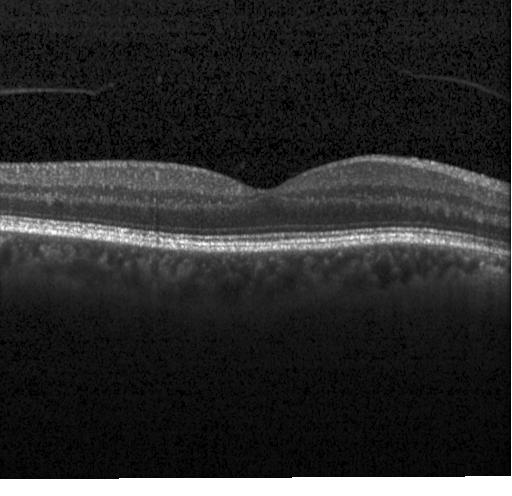

OCT B-scan — Macular OCT: no evidence of choroidal neovascularization, diabetic macular edema, or drusen.